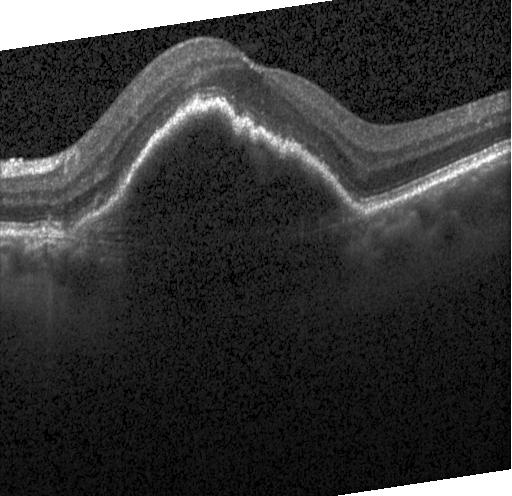
Spectral-domain OCT · Heidelberg Spectralis · retinal OCT B-scan.
The scan shows a choroidal neovascular membrane.